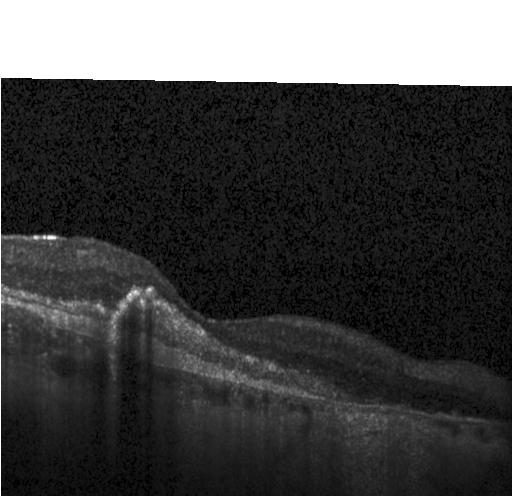 Macular OCT demonstrating CNV.